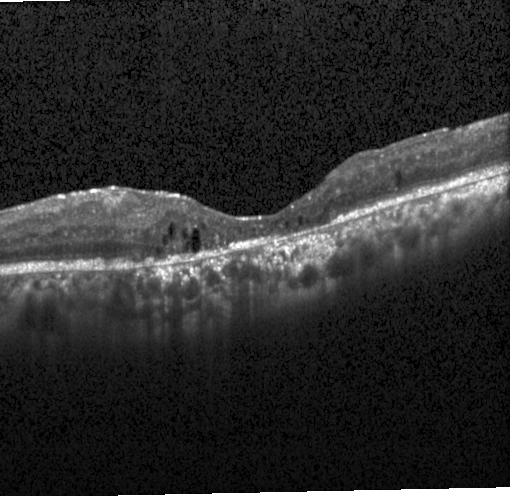

Heidelberg Spectralis, optical coherence tomography scan, spectral-domain OCT. Impression: CNV.